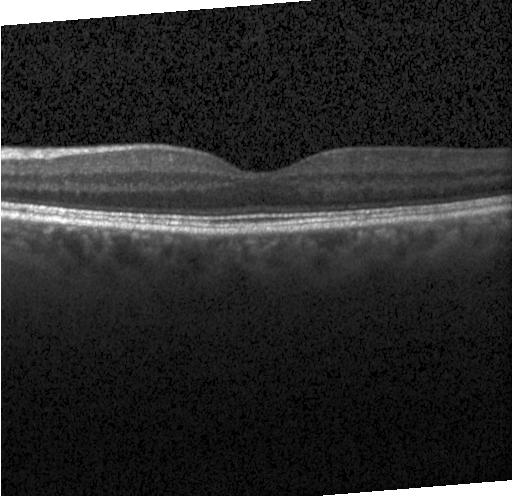

OCT B-scan showing no choroidal neovascularization, diabetic macular edema, or drusen.